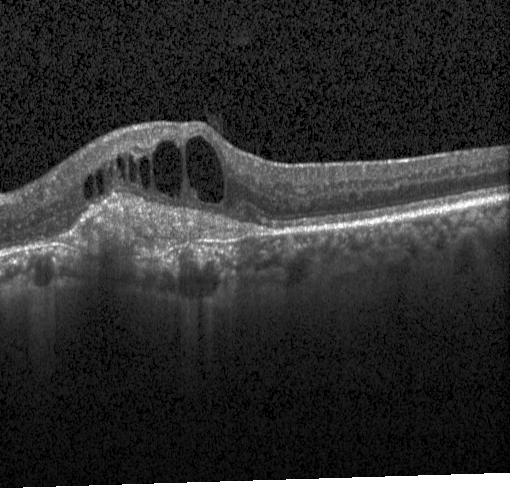
Centered on the fovea · retinal OCT cross-section · acquired on a Heidelberg Spectralis · spectral-domain OCT
This B-scan demonstrates a choroidal neovascular membrane.